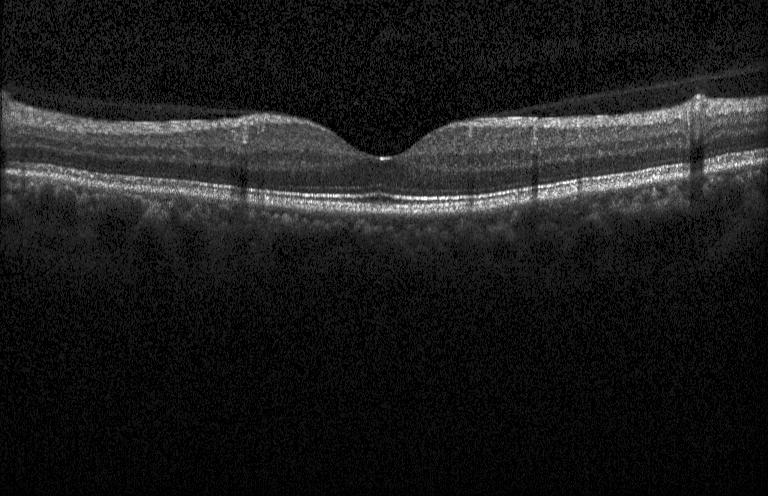

Macular OCT: neither choroidal neovascularization, diabetic macular edema, nor drusen.